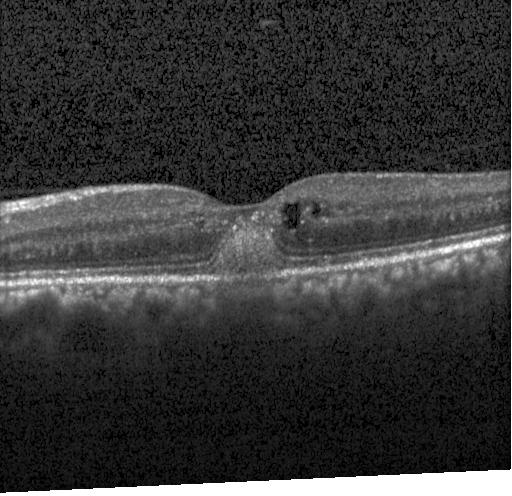
Spectral-domain OCT; centered on the fovea; retinal OCT cross-section — Diagnosis: a choroidal neovascular membrane.